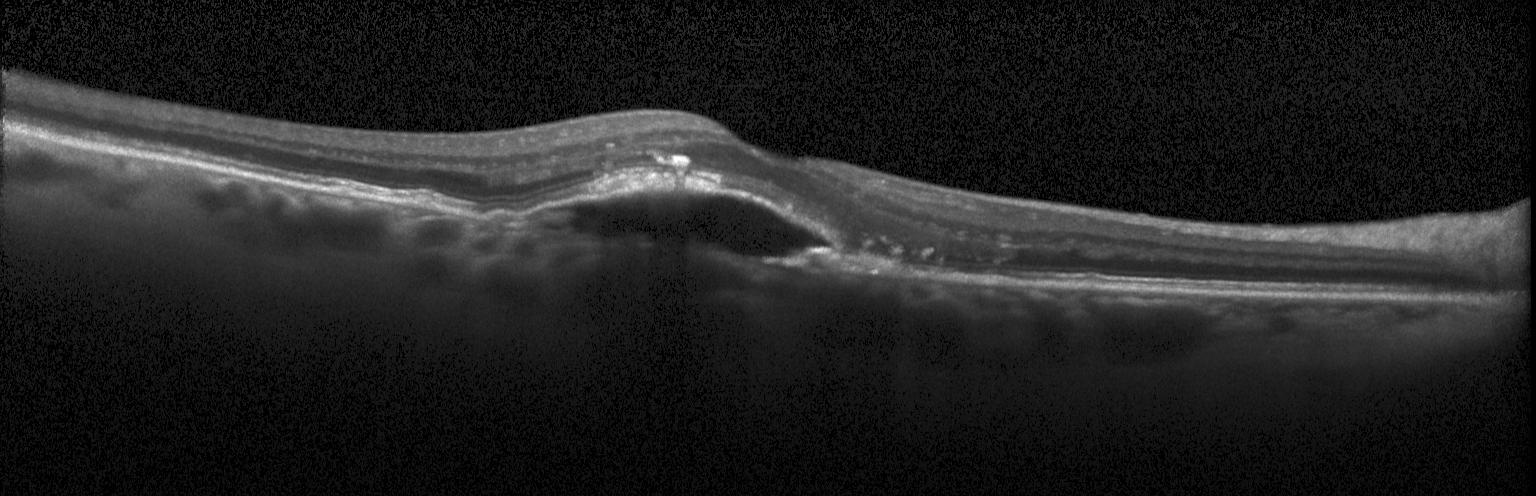

OCT scan showing choroidal neovascularization (CNV).